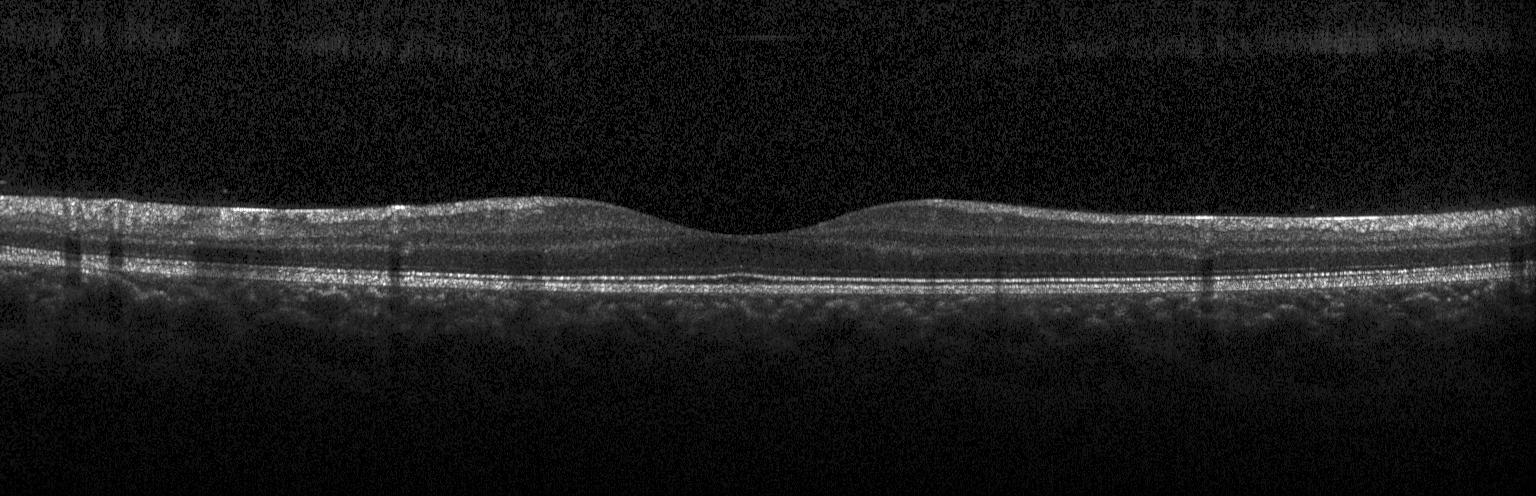

Optical coherence tomography scan.
Diagnosis: no choroidal neovascularization, no diabetic macular edema, and no drusen.